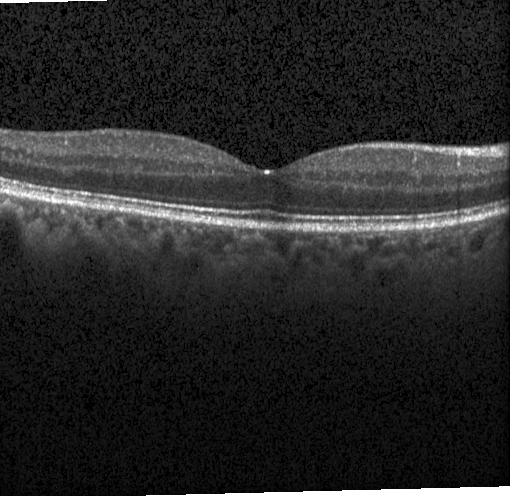
OCT finding: no CNV, DME, or drusen.